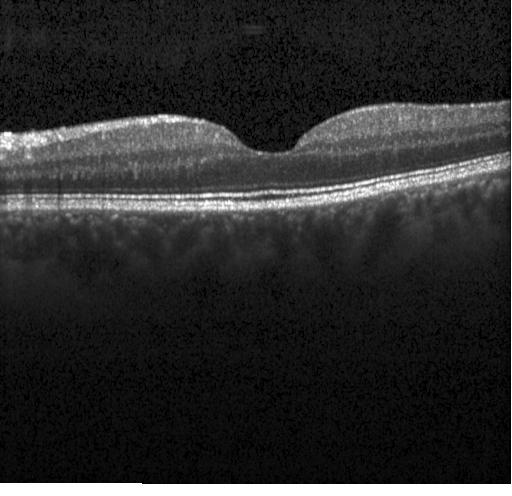

OCT B-scan.
Finding: no evidence of choroidal neovascularization, diabetic macular edema, or drusen.